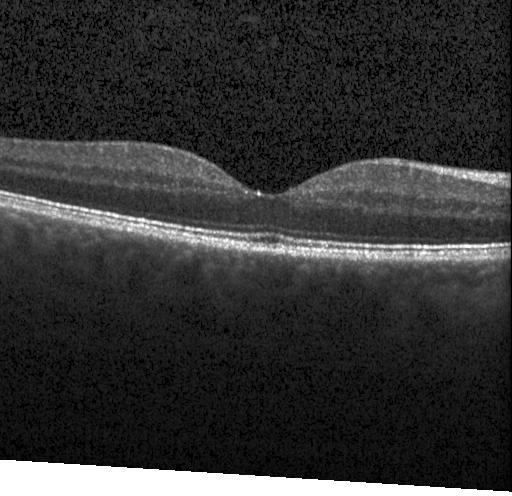 Spectral-domain OCT B-scan: no evidence of choroidal neovascularization, diabetic macular edema, or drusen.